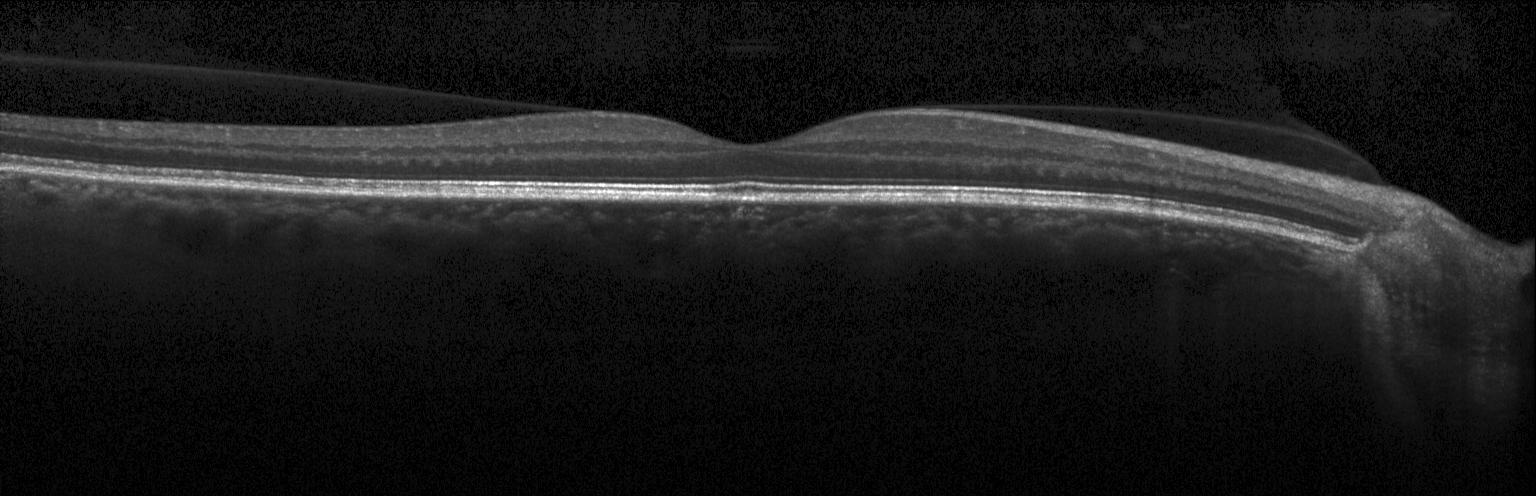 Horizontal scan through the fovea · SD-OCT · optical coherence tomography scan
Diagnosis: no evidence of choroidal neovascularization, diabetic macular edema, or drusen.